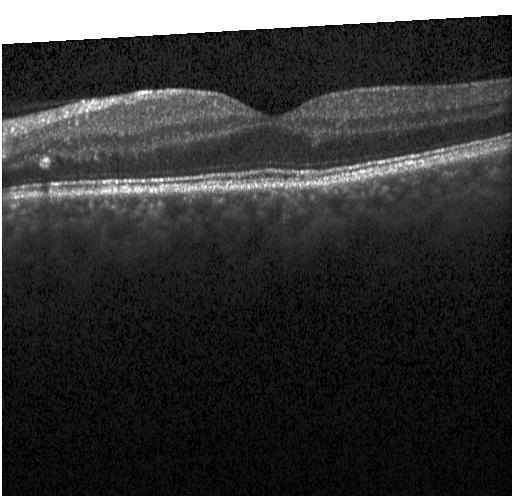

Retinal OCT B-scan, Heidelberg Spectralis OCT system. Diagnosis: no choroidal neovascularization, diabetic macular edema, or drusen.